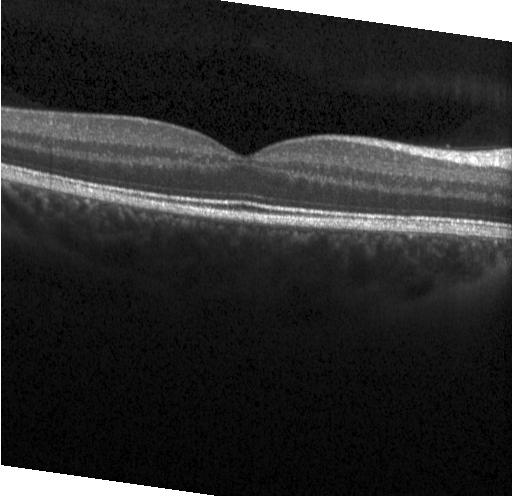 Impression: neither choroidal neovascularization, diabetic macular edema, nor drusen.